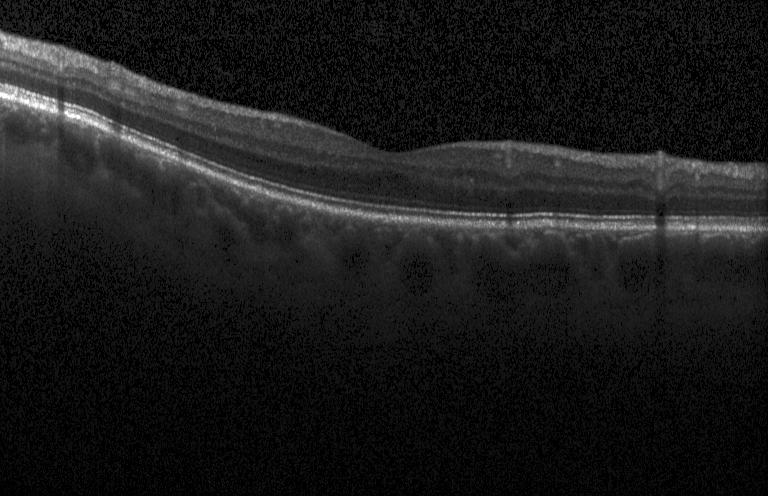 OCT B-scan.
This B-scan demonstrates no CNV, no DME, and no drusen.